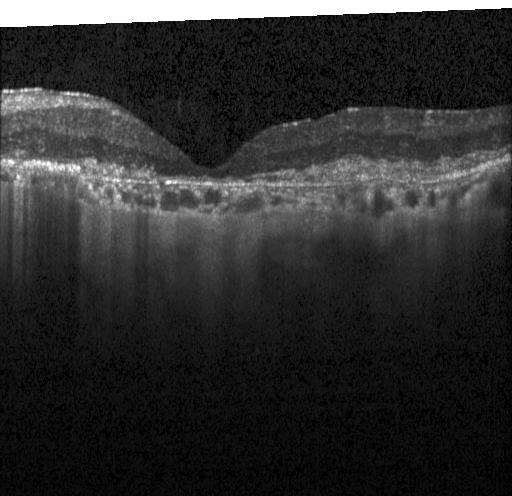
Impression: a choroidal neovascular membrane.